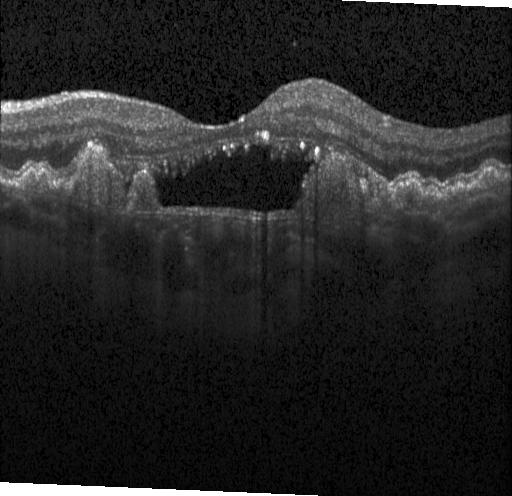 Retinal OCT cross-section, Heidelberg Spectralis OCT system.
OCT finding: a choroidal neovascular membrane.